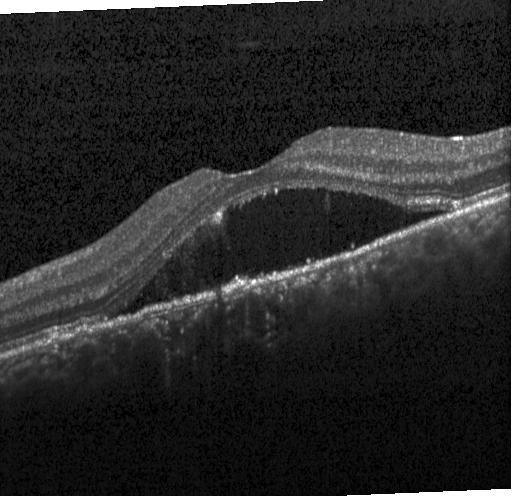
OCT finding: a choroidal neovascular membrane.